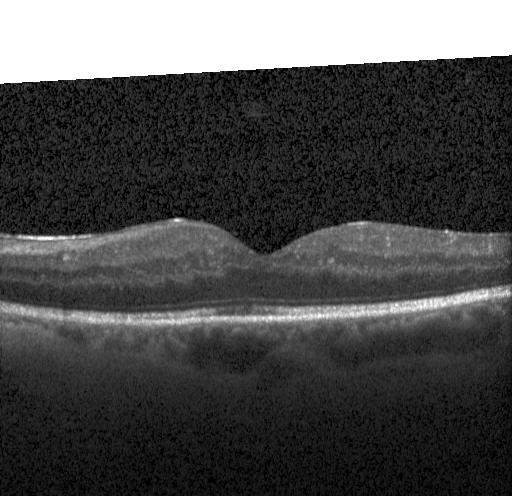
Spectral-domain optical coherence tomography. Optical coherence tomography scan.
Finding: diabetic macular edema.